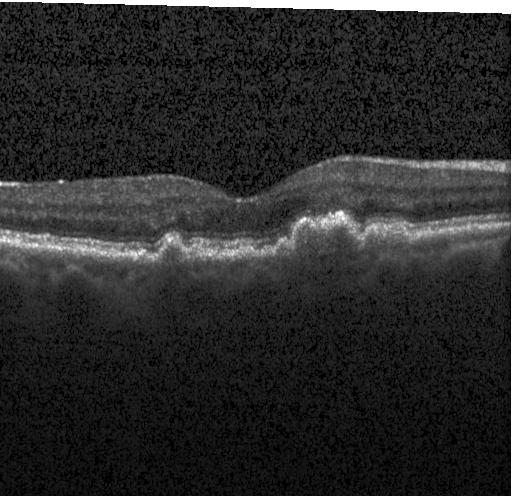

Instrument: Heidelberg Spectralis, horizontal scan through the fovea, optical coherence tomography scan.
Impression: sub-RPE drusenoid deposits.